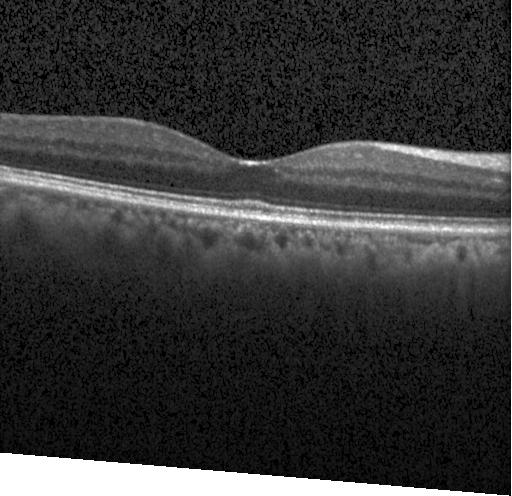

Through the macula, OCT B-scan, SD-OCT. Diagnosis: no choroidal neovascularization, diabetic macular edema, or drusen.